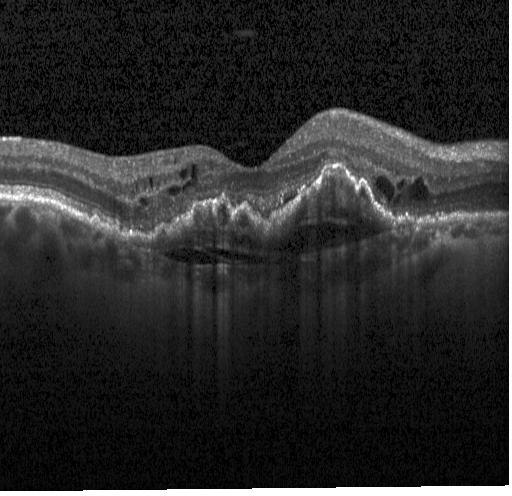 Optical coherence tomography scan. Assessment: CNV.